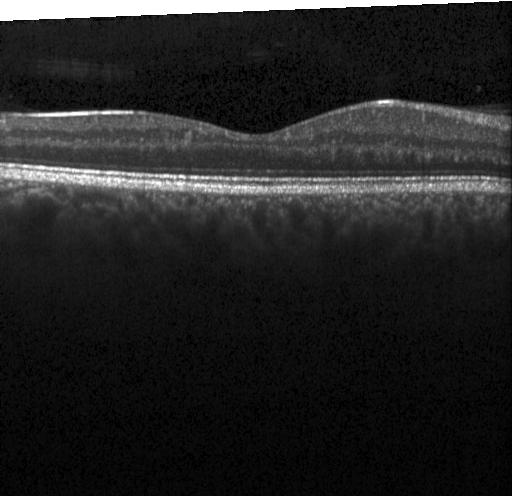

Spectral-domain optical coherence tomography. Retinal OCT cross-section.
Finding: no evidence of choroidal neovascularization, diabetic macular edema, or drusen.